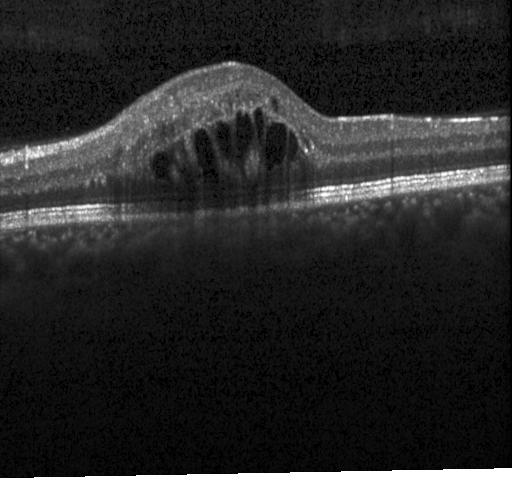
Retinal OCT cross-section — Finding: diabetic macular edema (DME).